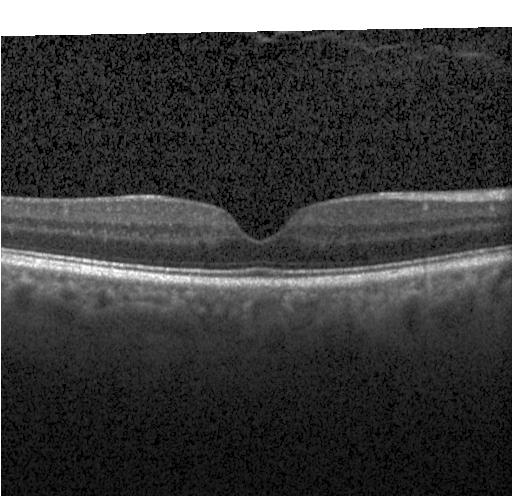 Acquired on a Heidelberg Spectralis · OCT B-scan · centered on the fovea. Impression: no choroidal neovascularization, diabetic macular edema, or drusen.